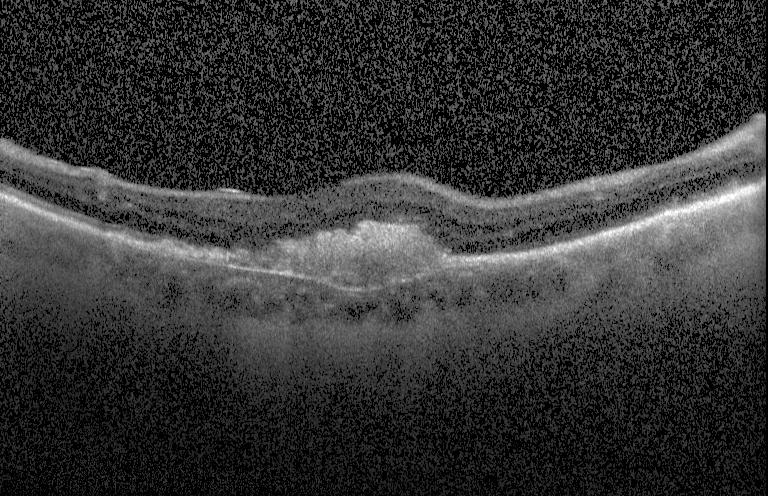

Acquired on a Heidelberg Spectralis. Spectral-domain optical coherence tomography. Centered on the fovea. Retinal OCT B-scan. This B-scan demonstrates a choroidal neovascular membrane.